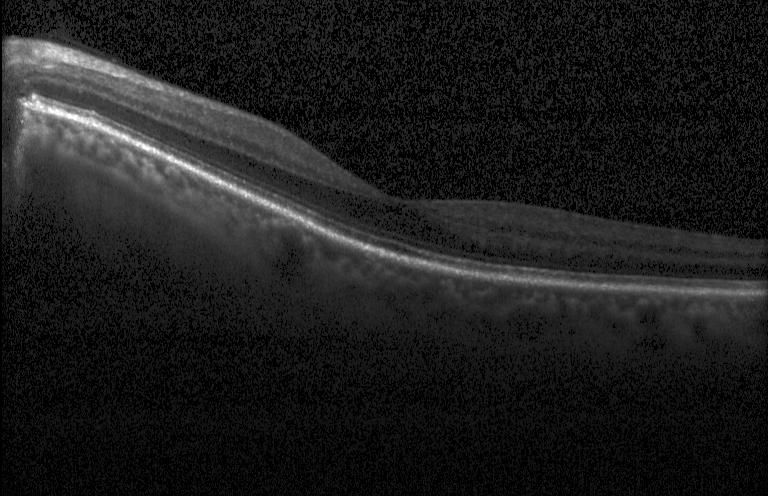

Optical coherence tomography B-scan
Assessment: neither choroidal neovascularization, diabetic macular edema, nor drusen.